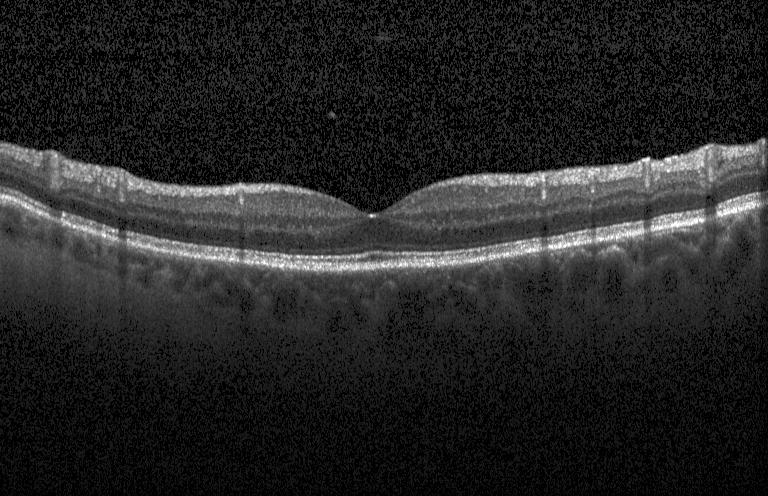

Horizontal scan through the fovea; retinal OCT cross-section — Impression: no evidence of CNV, DME, or drusen.